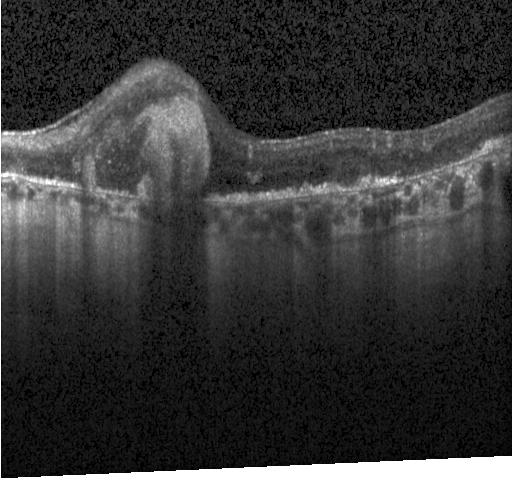

Macular OCT: choroidal neovascularization.